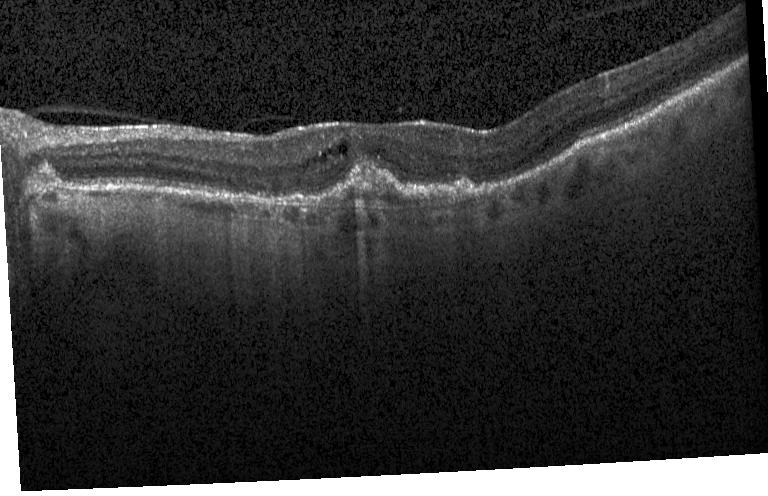 Spectral-domain OCT B-scan: a choroidal neovascular membrane.